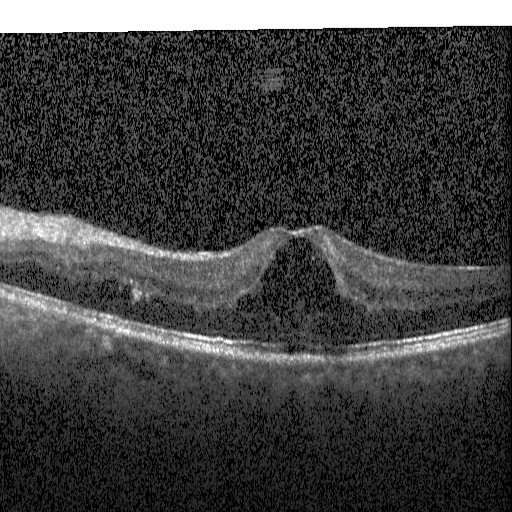 OCT B-scan — Diagnosis: DME.